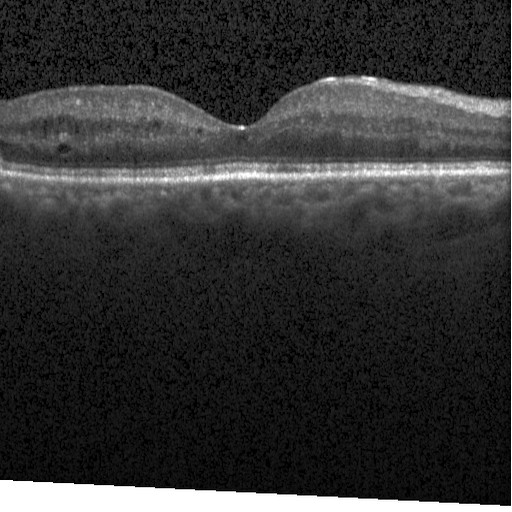 OCT B-scan.
DME.